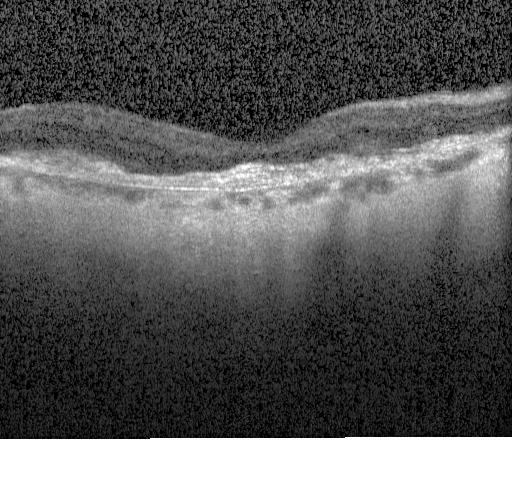
Through the macula · optical coherence tomography B-scan — Finding: a choroidal neovascular membrane.